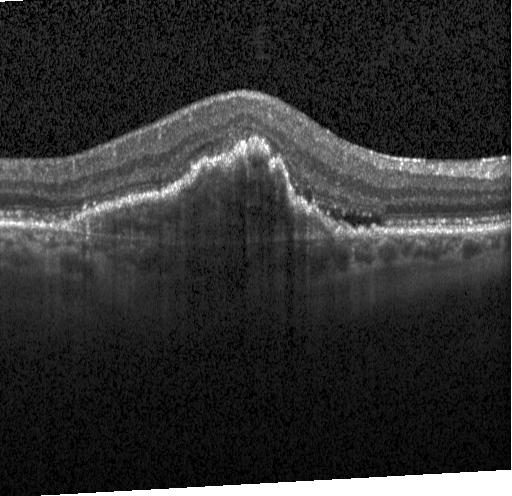 OCT line scan.
The scan shows choroidal neovascularization (CNV).